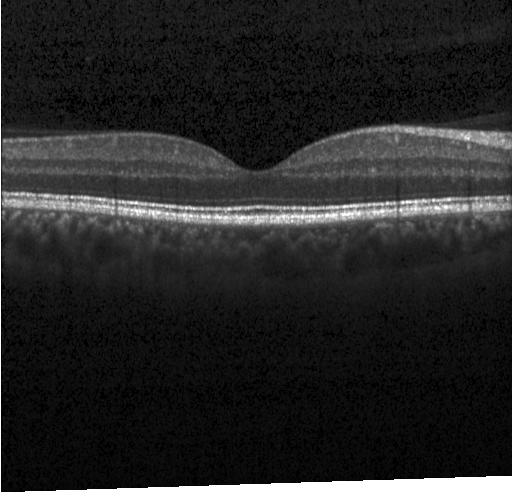

Acquired on a Heidelberg Spectralis · through the macula · spectral-domain optical coherence tomography · optical coherence tomography scan. Diagnosis: no CNV, no DME, and no drusen.